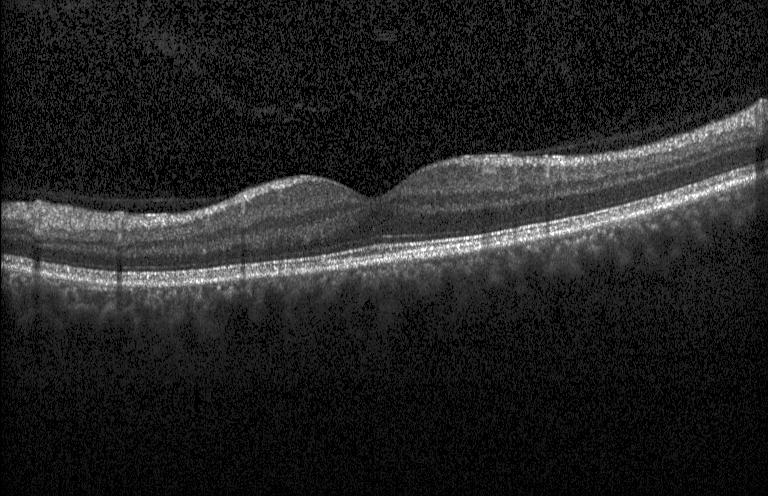
Retinal OCT cross-section showing neither CNV, DME, nor drusen.